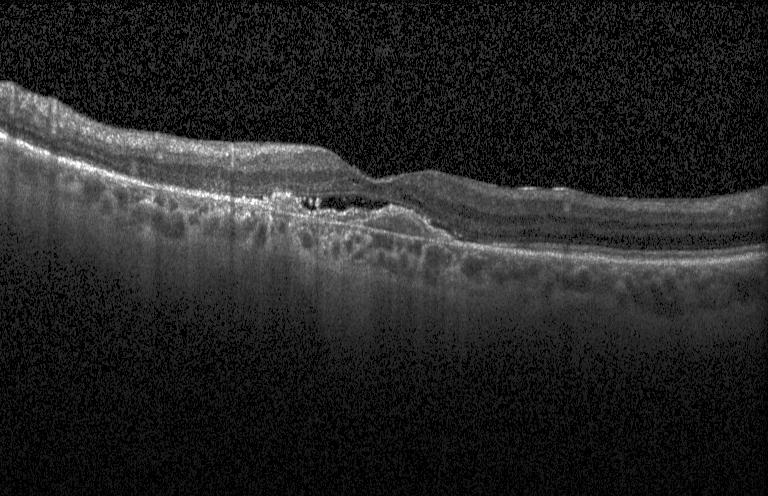
Retinal OCT cross-section; centered on the fovea. Diagnosis: CNV.